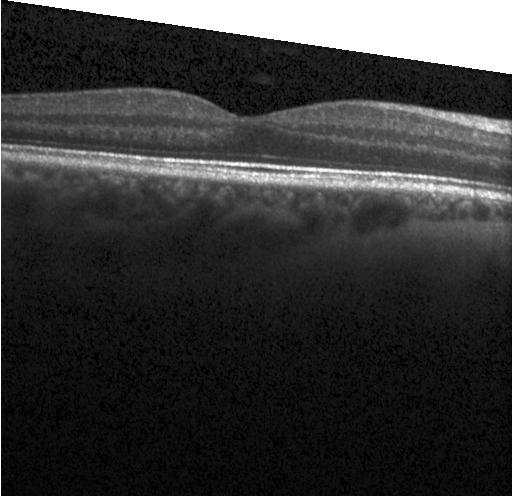
Optical coherence tomography B-scan; acquired on a Heidelberg Spectralis — Diagnosis: neither CNV, DME, nor drusen.